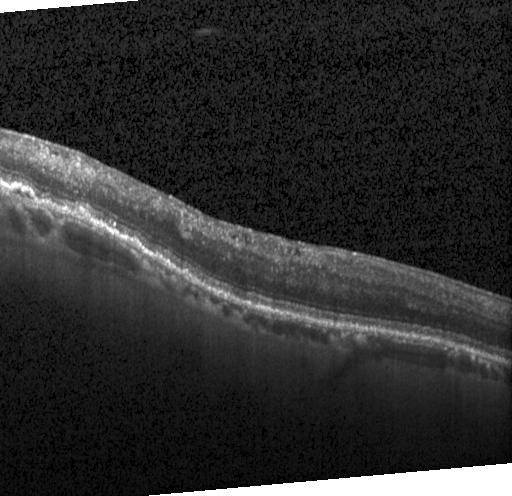
OCT line scan. Dx: choroidal neovascularization (CNV).